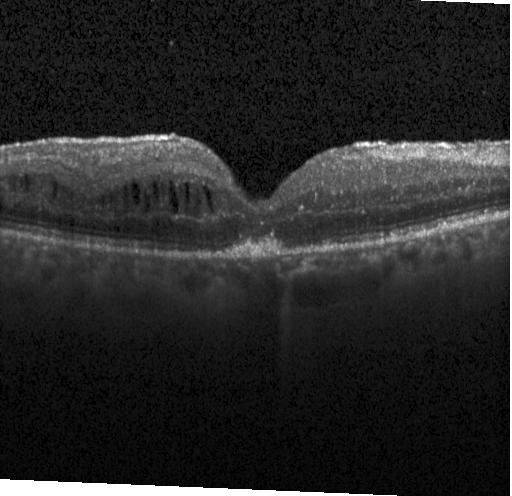
Diagnosis: diabetic macular edema (DME).